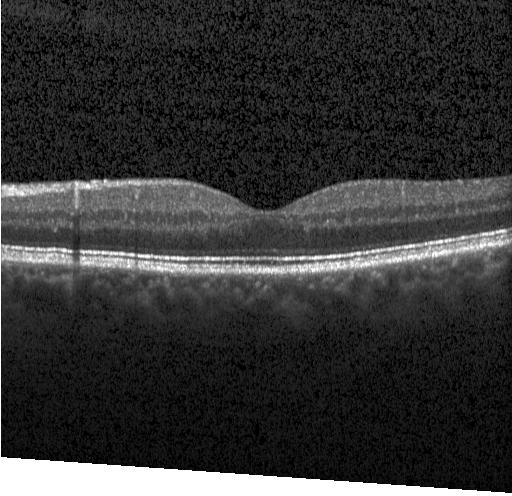 Optical coherence tomography B-scan.
OCT finding: no evidence of choroidal neovascularization, diabetic macular edema, or drusen.